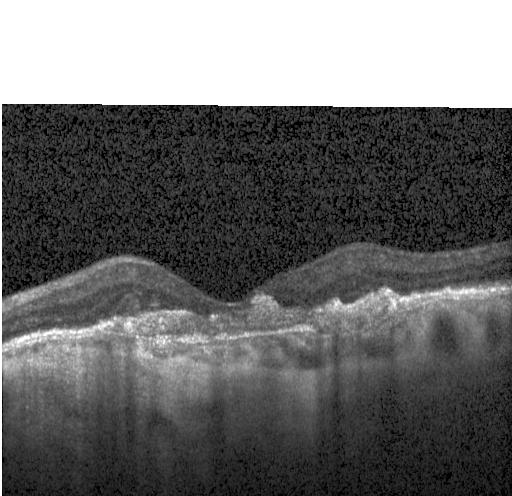

Retinal OCT cross-section.
Diagnosis: choroidal neovascularization.